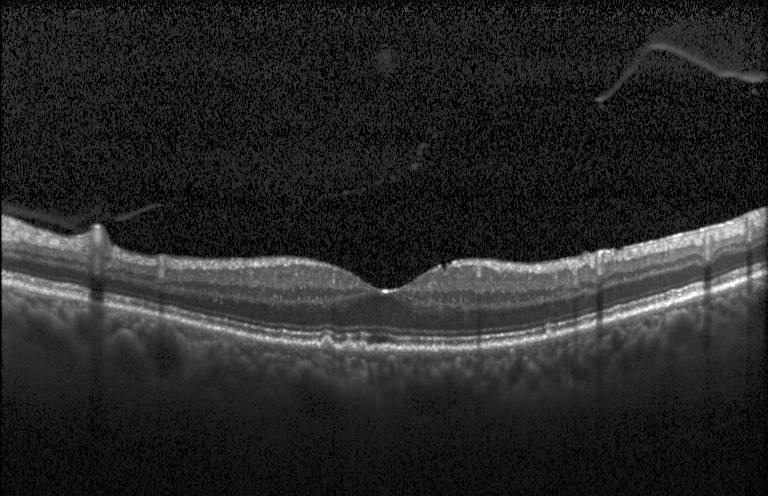

OCT line scan, spectral-domain optical coherence tomography. Finding: drusen.